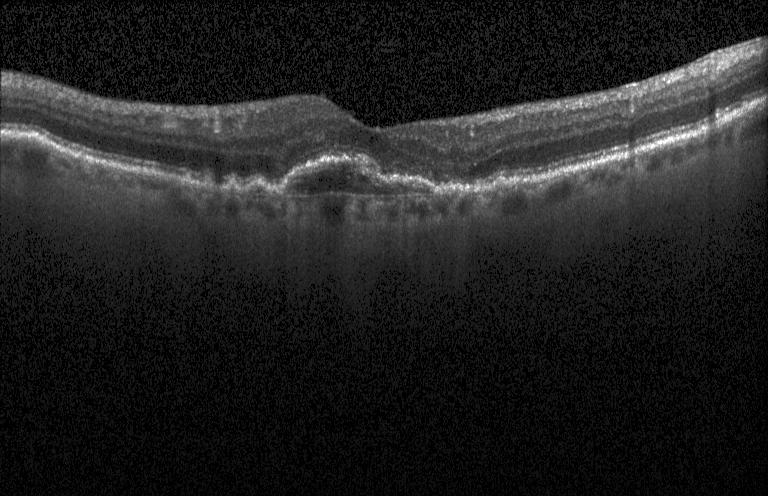 Instrument: Heidelberg Spectralis, horizontal scan through the fovea, retinal OCT B-scan. A choroidal neovascular membrane.